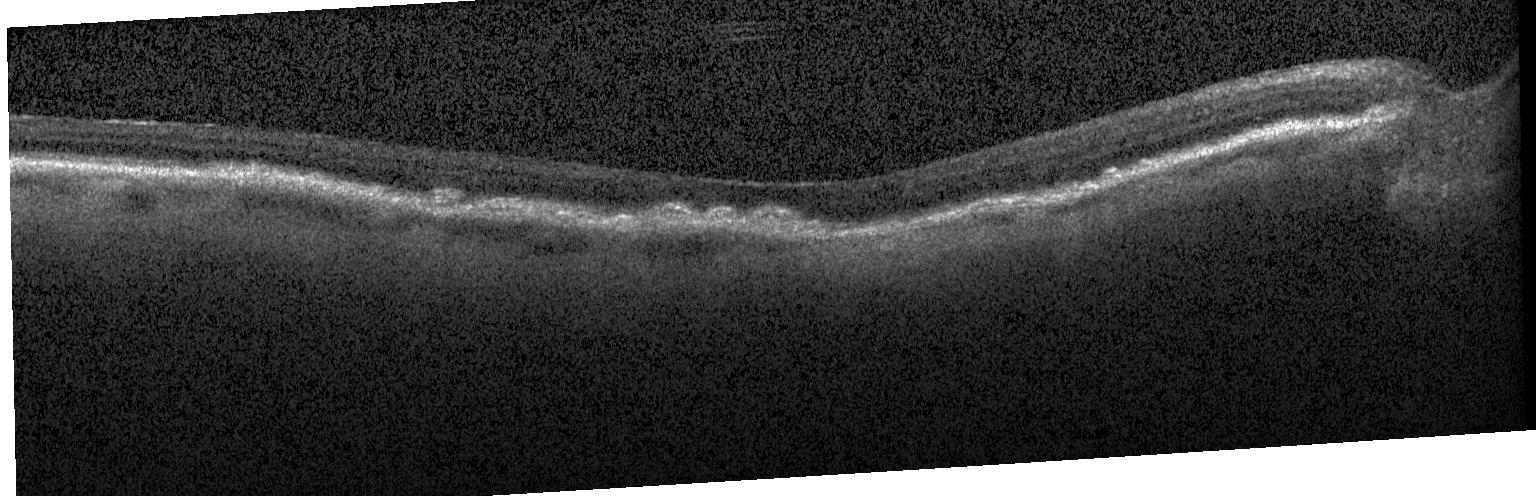
Optical coherence tomography B-scan · spectral-domain OCT. The scan shows choroidal neovascularization.